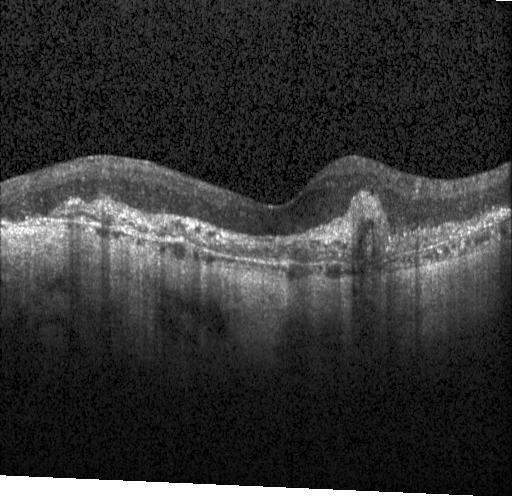 Retinal OCT B-scan.
Finding: a choroidal neovascular membrane.